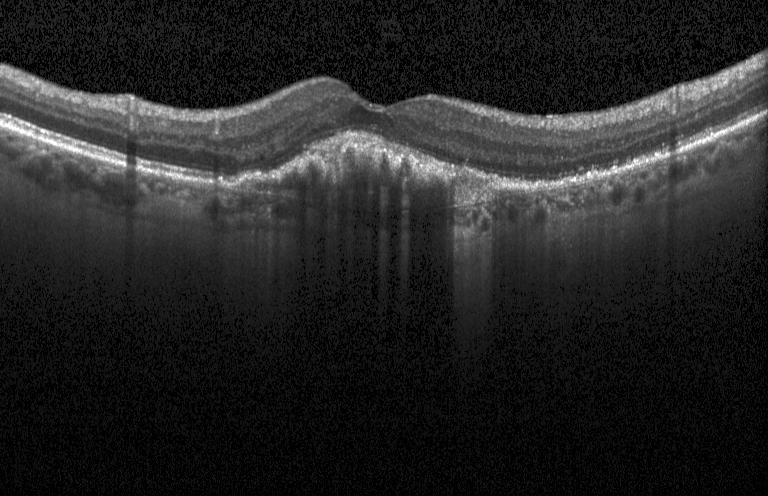 OCT finding: CNV.